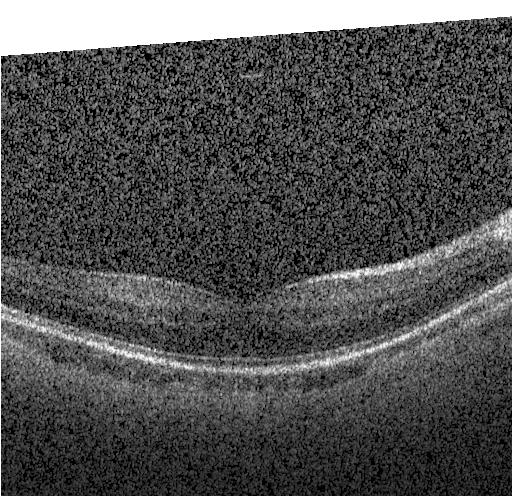

Acquired on a Heidelberg Spectralis · retinal OCT B-scan · horizontal scan through the fovea · spectral-domain optical coherence tomography.
This B-scan demonstrates neither CNV, DME, nor drusen.